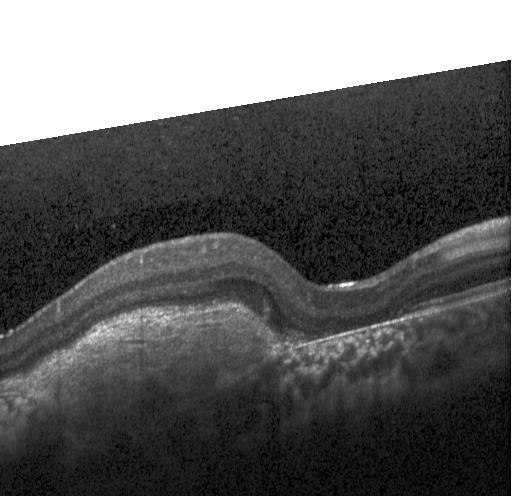 Finding: choroidal neovascularization.